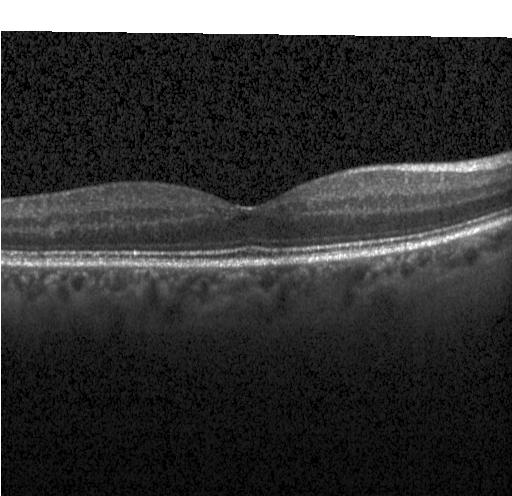 The scan shows no evidence of choroidal neovascularization, diabetic macular edema, or drusen.